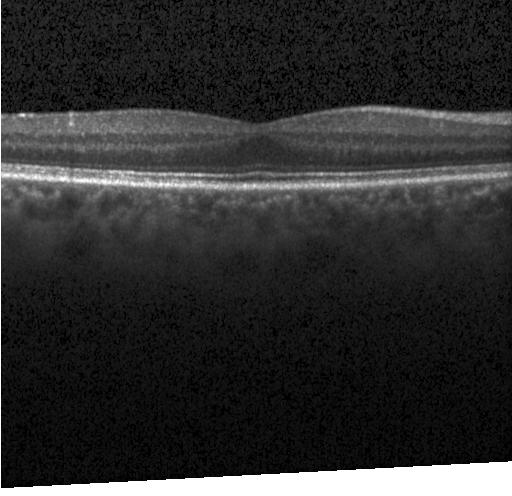

Macular OCT: no choroidal neovascularization, diabetic macular edema, or drusen.